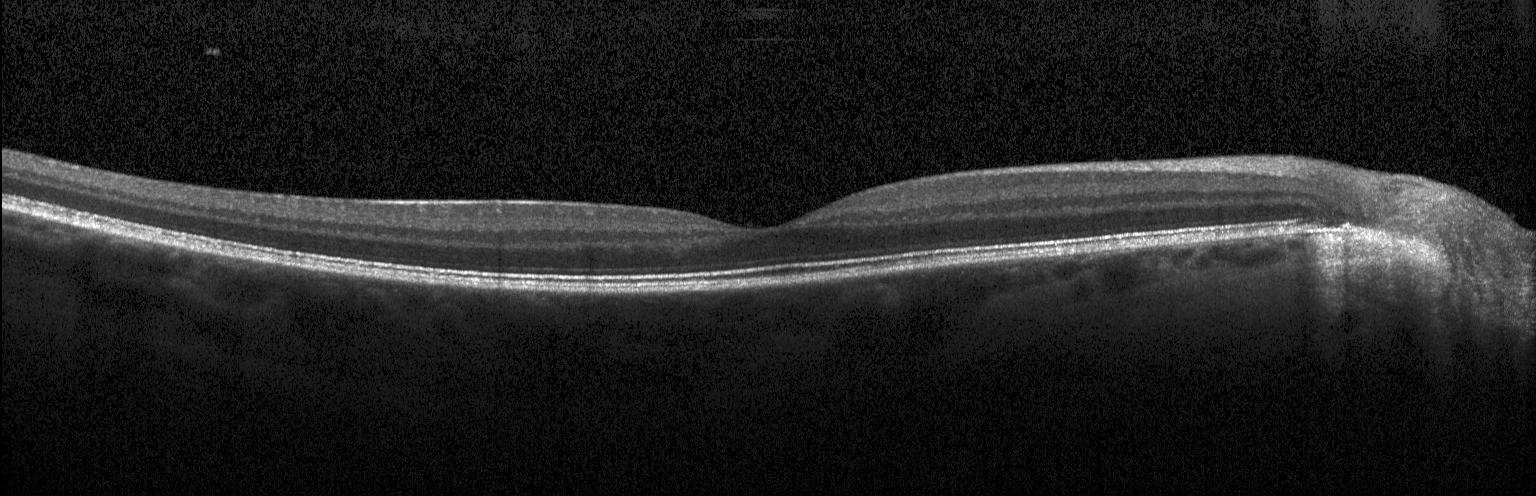 This B-scan demonstrates no choroidal neovascularization, diabetic macular edema, or drusen.